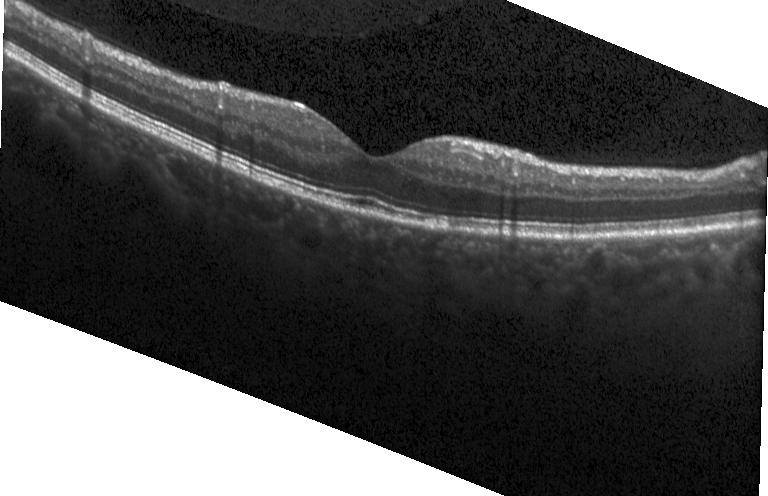
Instrument: Heidelberg Spectralis, spectral-domain optical coherence tomography, centered on the fovea, retinal OCT B-scan.
Impression: no choroidal neovascularization, diabetic macular edema, or drusen.